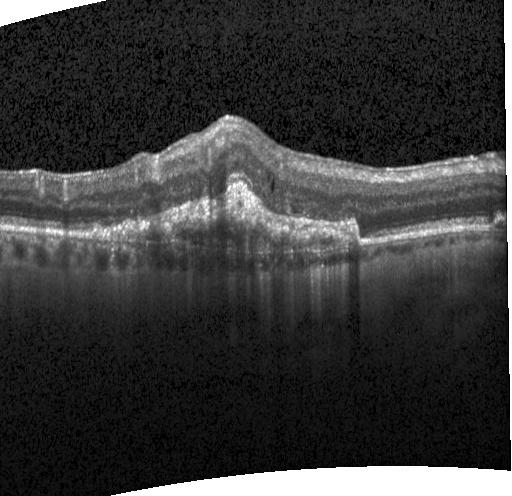

Spectral-domain optical coherence tomography; horizontal scan through the fovea; retinal OCT B-scan
Finding: choroidal neovascularization.